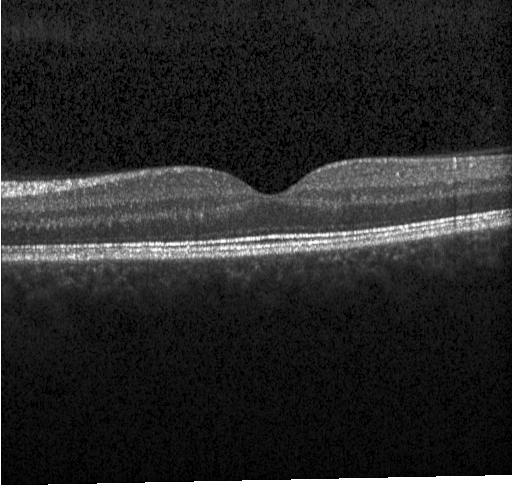 Optical coherence tomography scan
Finding: no choroidal neovascularization, diabetic macular edema, or drusen.